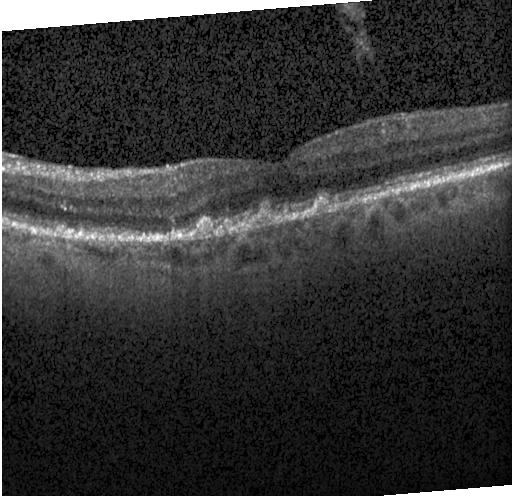 OCT line scan, fovea-centered
Dx: multiple drusen.